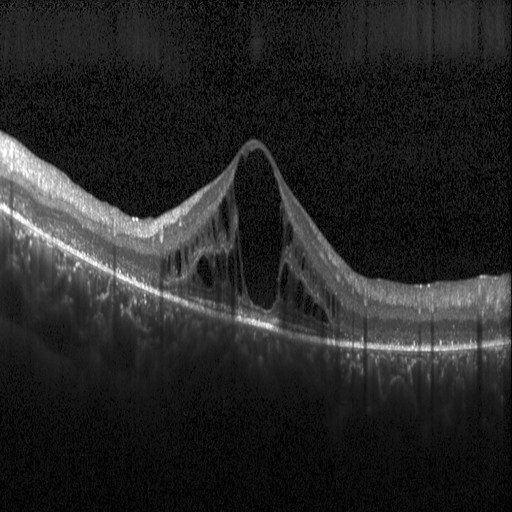

Impression: diabetic macular edema.